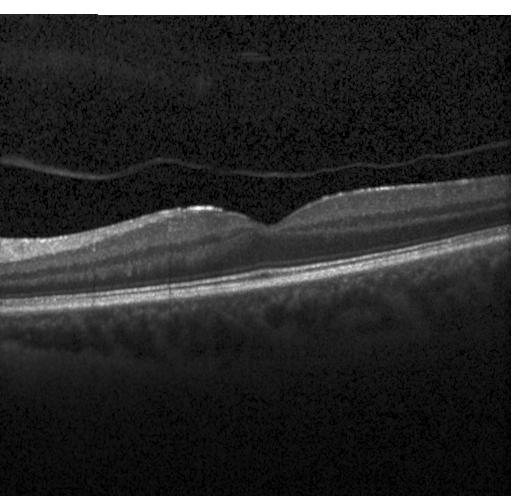 Horizontal scan through the fovea, OCT line scan — The scan shows no evidence of choroidal neovascularization, diabetic macular edema, or drusen.